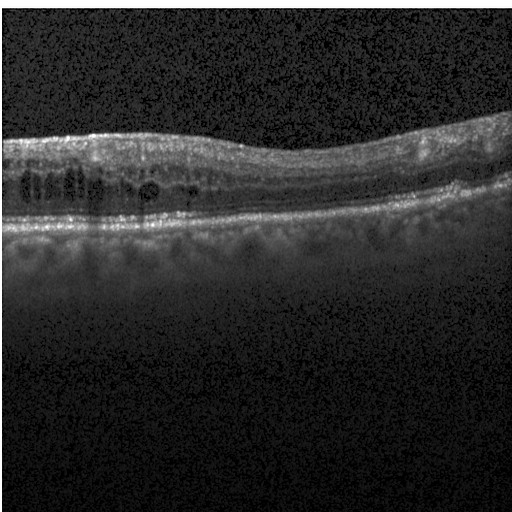
Spectral-domain optical coherence tomography, optical coherence tomography scan
Assessment: diabetic macular edema.